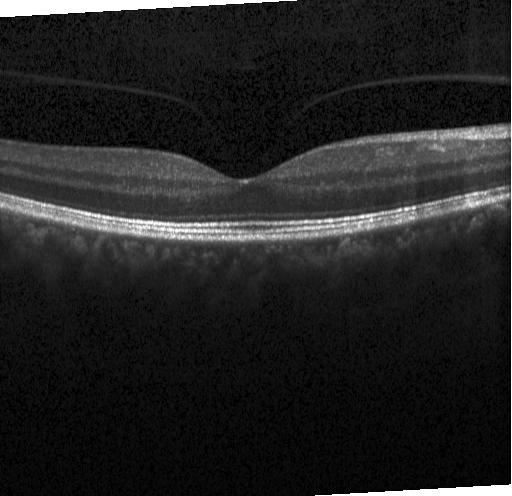

Dx: no choroidal neovascularization, no diabetic macular edema, and no drusen.